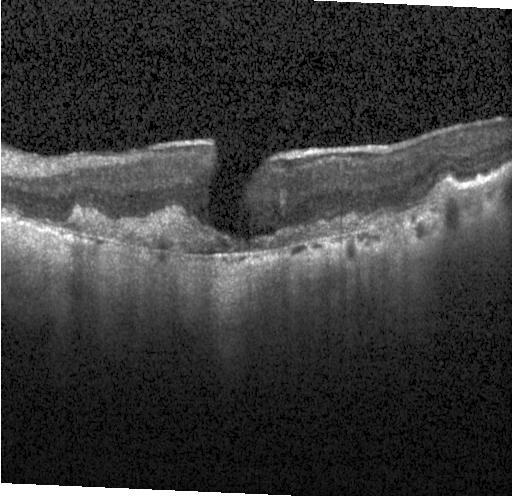

Optical coherence tomography scan; SD-OCT
OCT finding: a choroidal neovascular membrane.